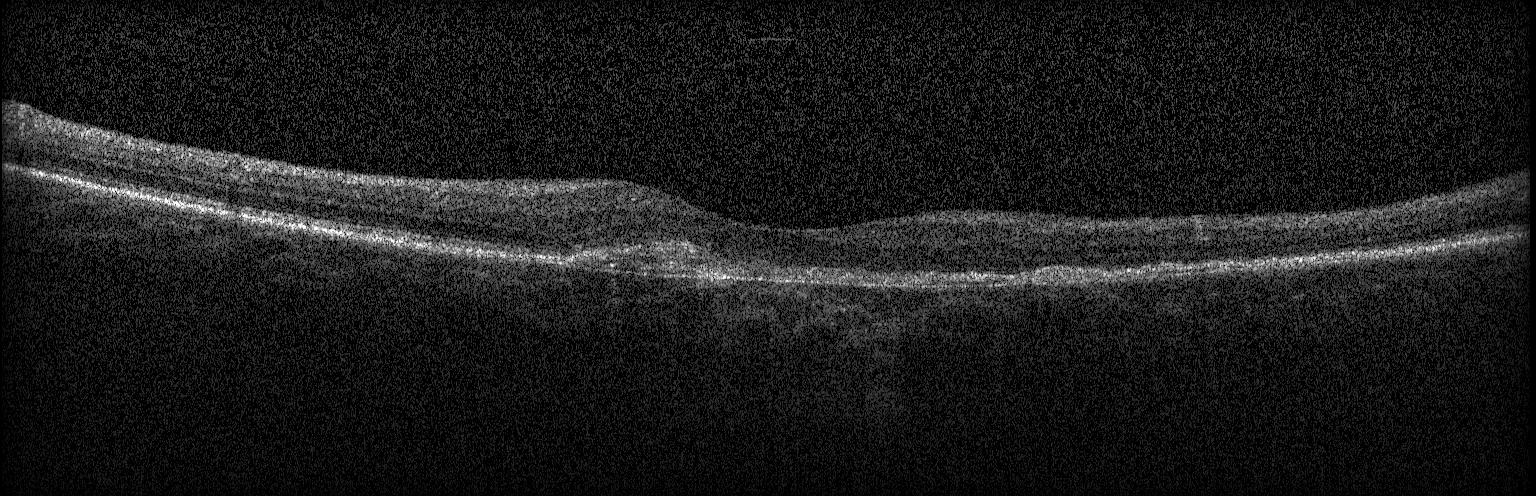
Macular OCT: a choroidal neovascular membrane.